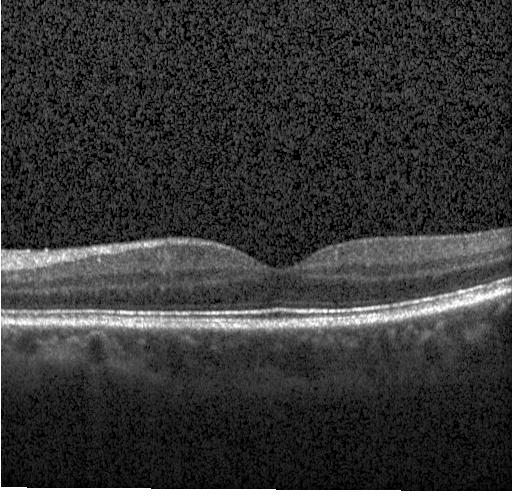 Retinal OCT cross-section.
Finding: no choroidal neovascularization, diabetic macular edema, or drusen.